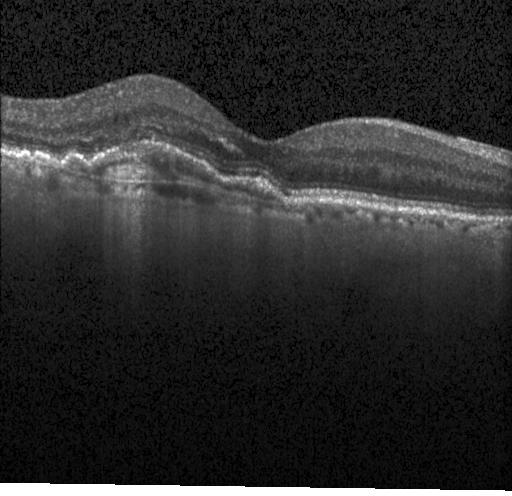
Macular OCT: CNV.